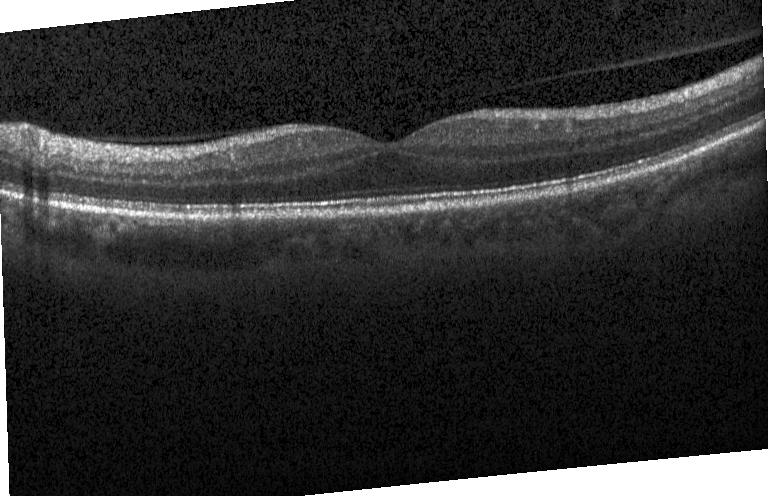

Optical coherence tomography B-scan. Through the macula. Acquired on a Heidelberg Spectralis. Spectral-domain optical coherence tomography. Assessment: no evidence of CNV, DME, or drusen.